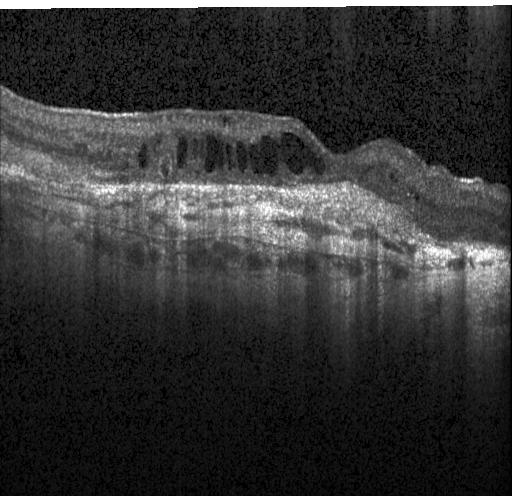 OCT line scan; spectral-domain optical coherence tomography; Heidelberg Spectralis
Macular OCT: choroidal neovascularization (CNV).